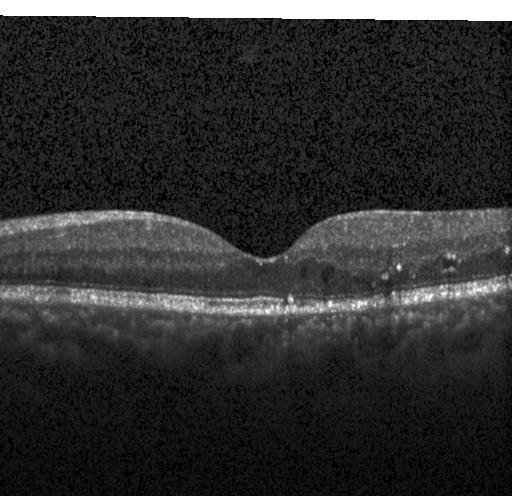

Heidelberg Spectralis. Fovea-centered. Optical coherence tomography scan
Finding: diabetic macular edema (DME).